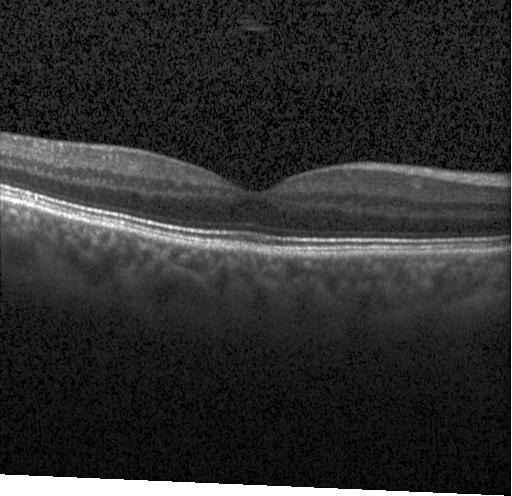

Acquired on a Heidelberg Spectralis, optical coherence tomography scan.
Assessment: no choroidal neovascularization, diabetic macular edema, or drusen.